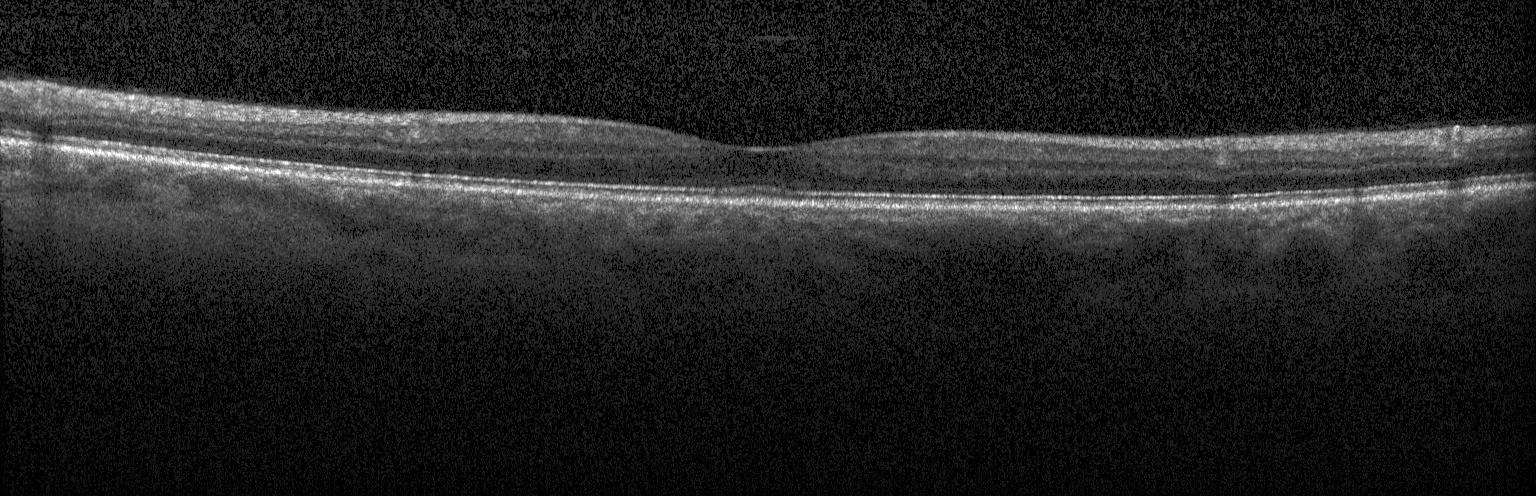
OCT B-scan · Heidelberg Spectralis · SD-OCT · macular scan
The scan shows no evidence of choroidal neovascularization, diabetic macular edema, or drusen.